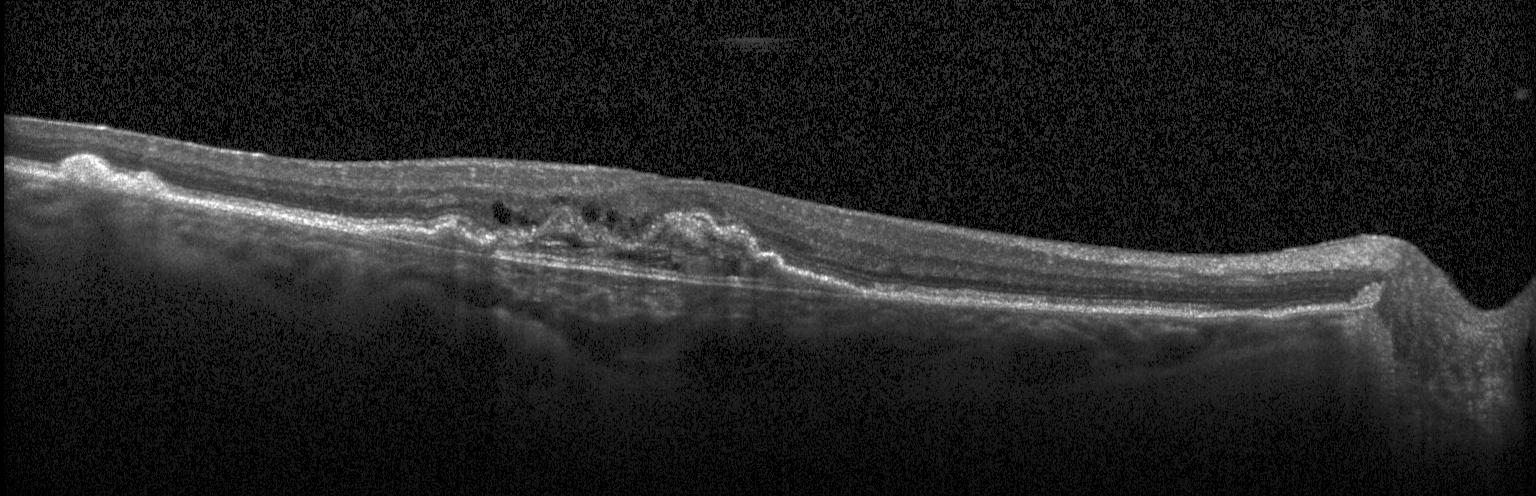

Retinal OCT cross-section. Dx: choroidal neovascularization (CNV).